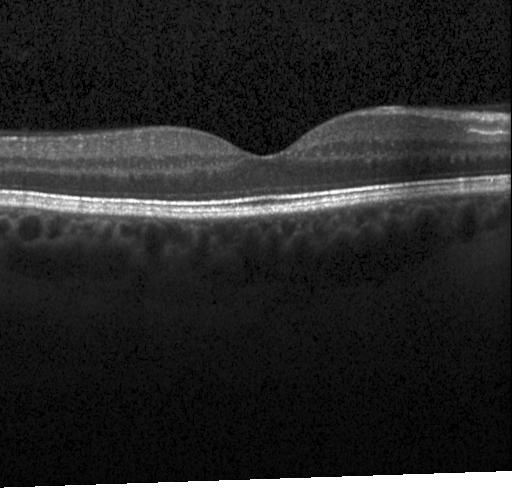
Diagnosis: no CNV, no DME, and no drusen.